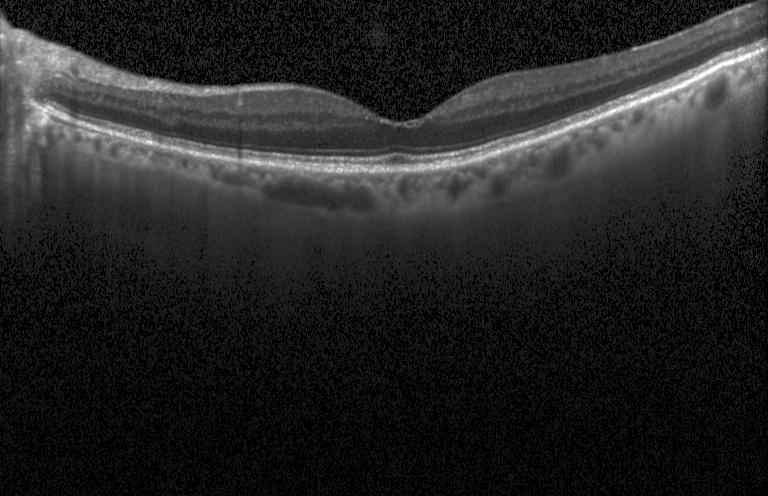

Dx: no evidence of choroidal neovascularization, diabetic macular edema, or drusen.